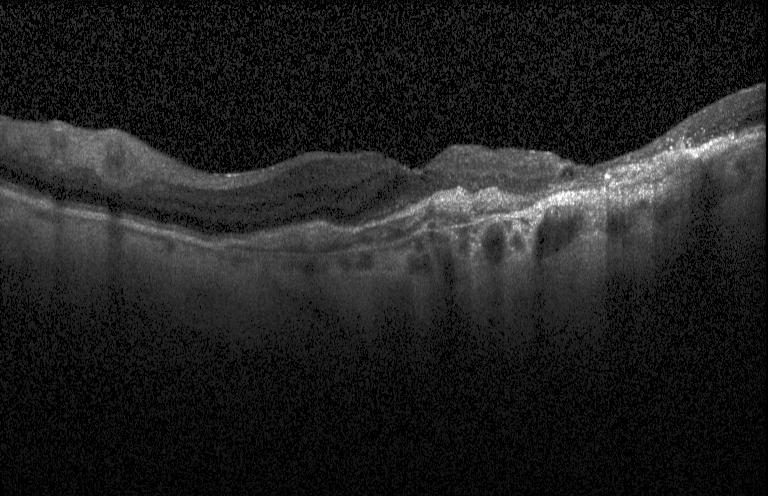

OCT B-scan, spectral-domain optical coherence tomography — Impression: a choroidal neovascular membrane.